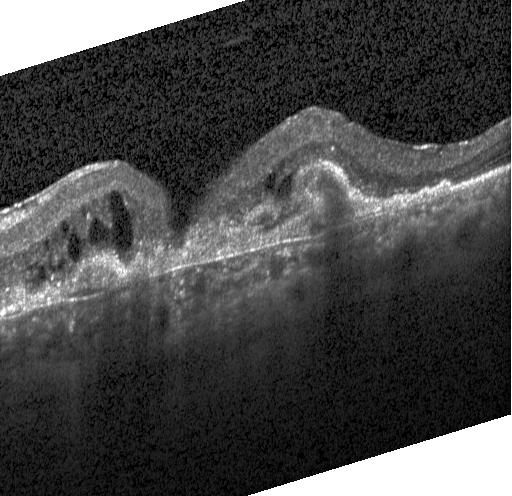
Optical coherence tomography B-scan
Choroidal neovascularization.